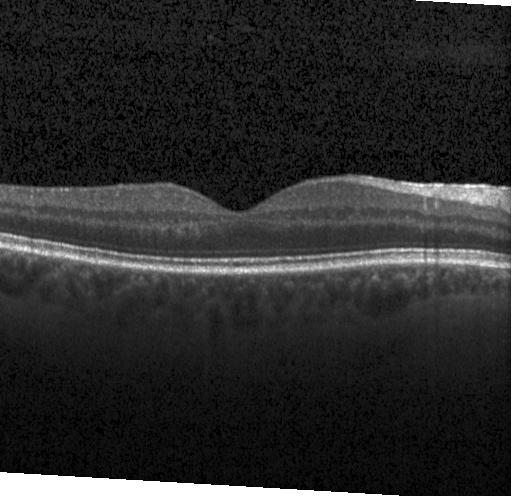

Diagnosis: no choroidal neovascularization, diabetic macular edema, or drusen.